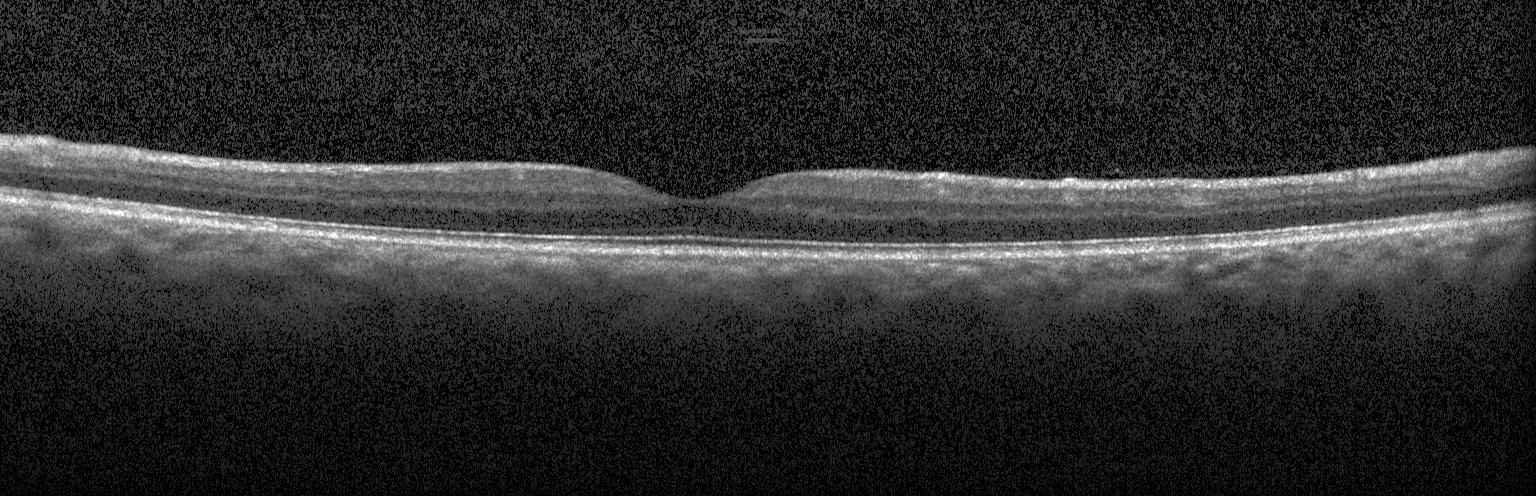
Finding: no evidence of choroidal neovascularization, diabetic macular edema, or drusen.